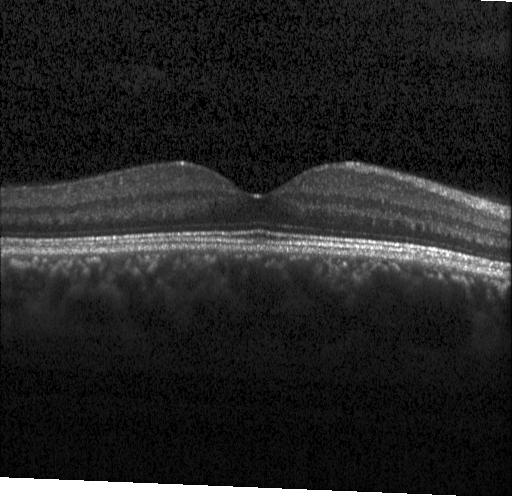
Diagnosis: no evidence of choroidal neovascularization, diabetic macular edema, or drusen.